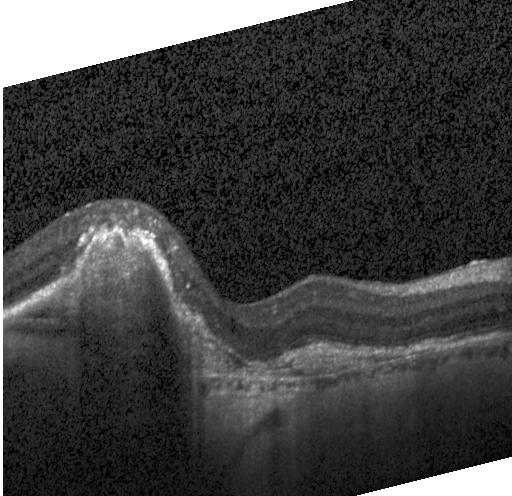

Heidelberg Spectralis. OCT B-scan
Dx: CNV.